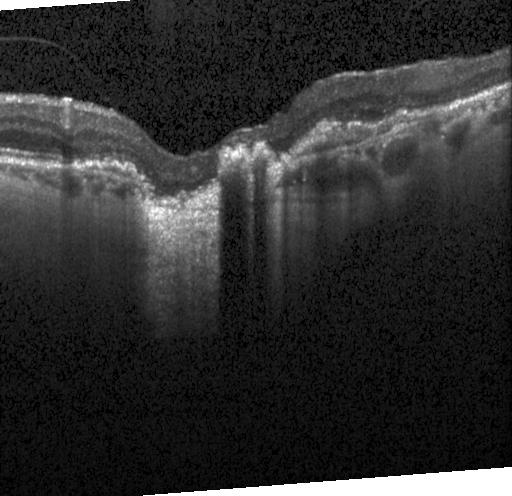 OCT B-scan.
OCT finding: choroidal neovascularization.